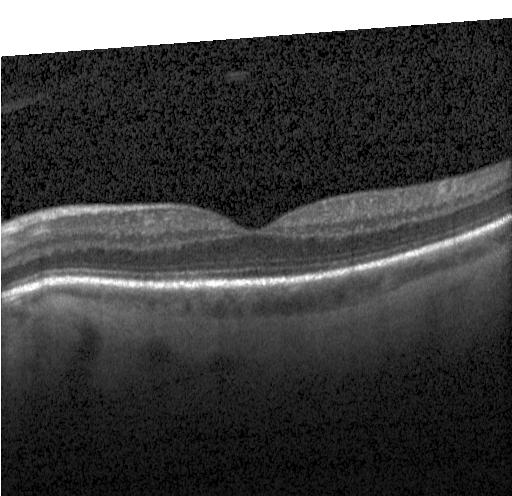
Diagnosis: no CNV, no DME, and no drusen.